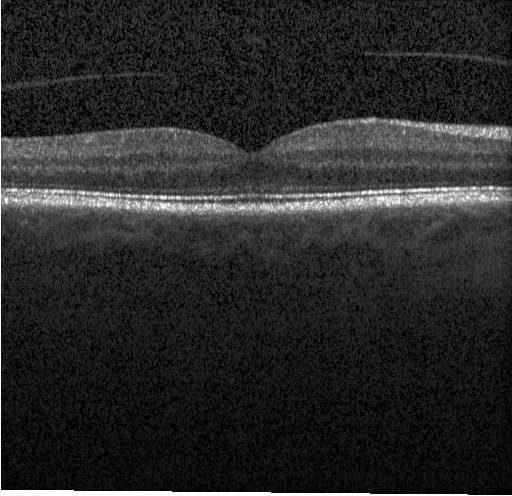

Retinal OCT cross-section · fovea-centered · acquired on a Heidelberg Spectralis · spectral-domain optical coherence tomography
No choroidal neovascularization, diabetic macular edema, or drusen.